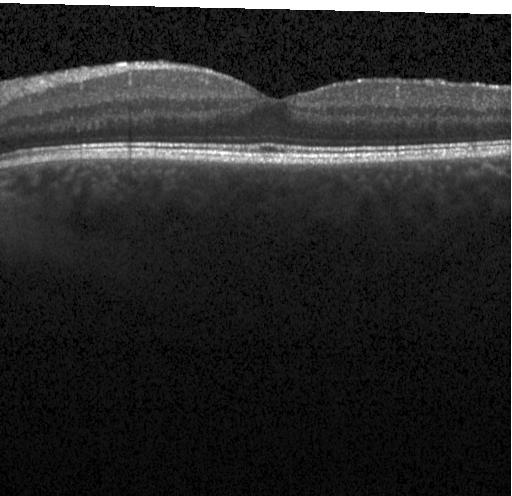
Macular OCT demonstrating no CNV, no DME, and no drusen.